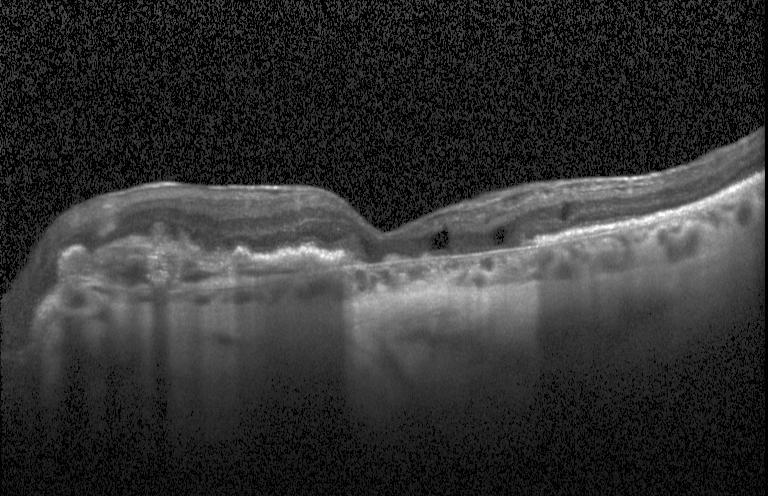

Impression: choroidal neovascularization (CNV).